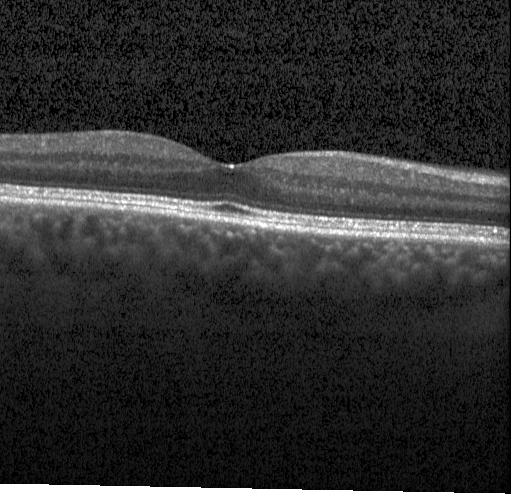
Dx: neither CNV, DME, nor drusen.